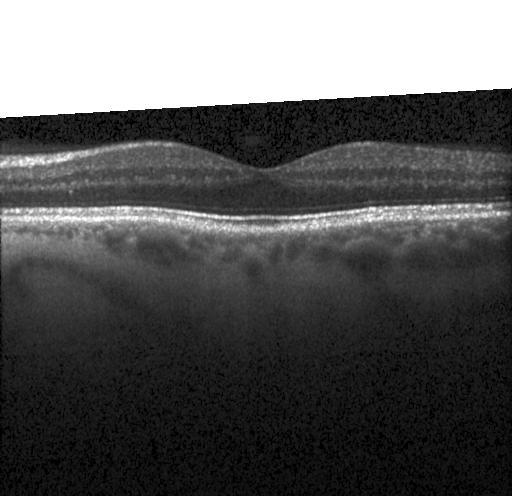

Centered on the fovea, instrument: Heidelberg Spectralis, OCT line scan — This B-scan demonstrates no CNV, DME, or drusen.